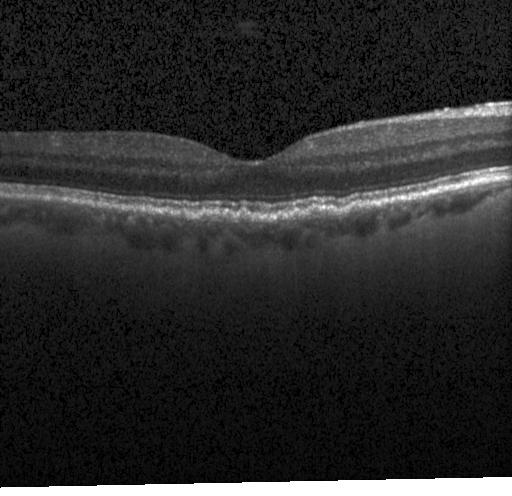
Optical coherence tomography scan. This B-scan demonstrates sub-RPE drusenoid deposits.